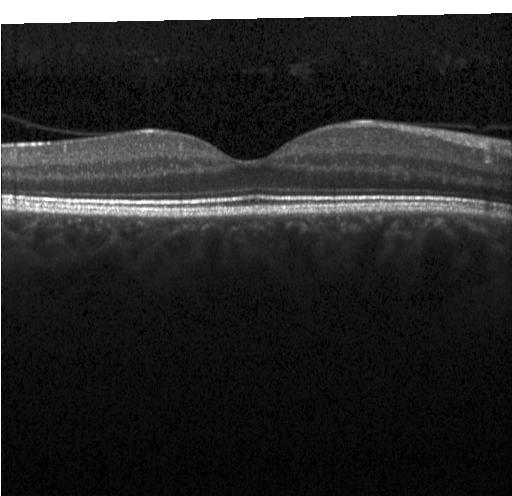 Retinal OCT B-scan; instrument: Heidelberg Spectralis.
The scan shows no evidence of choroidal neovascularization, diabetic macular edema, or drusen.